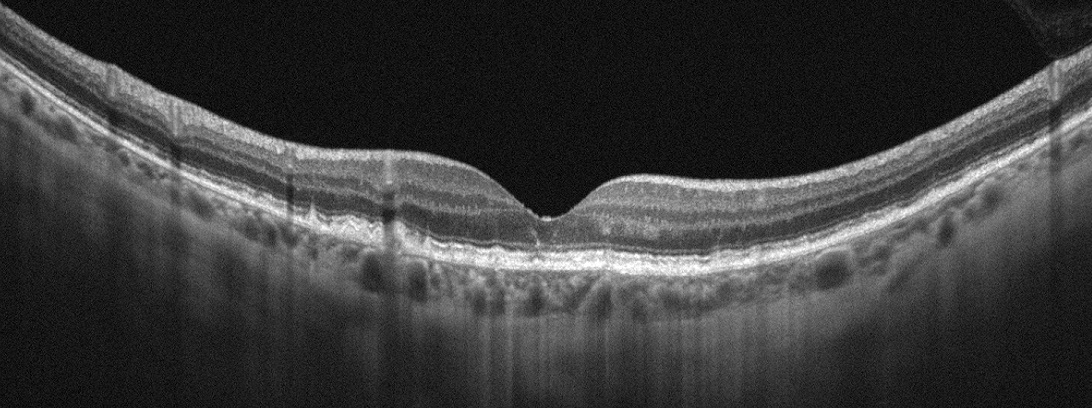

This B-scan demonstrates AMD.